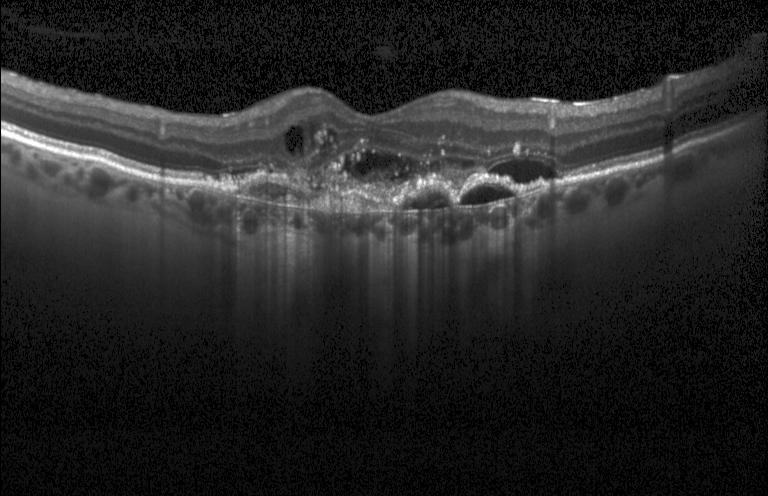

Retinal OCT cross-section; Heidelberg Spectralis OCT system — Diagnosis: CNV.